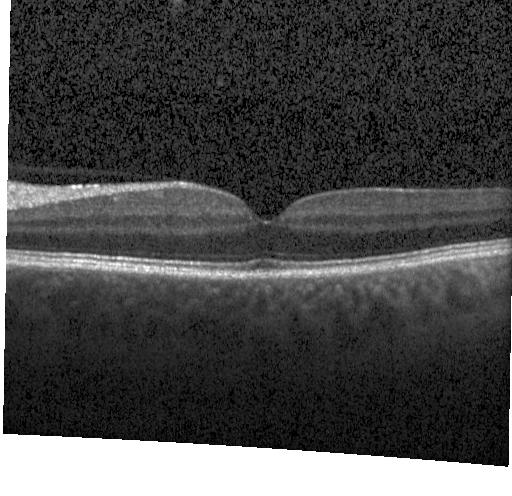 Diagnosis: no evidence of choroidal neovascularization, diabetic macular edema, or drusen.